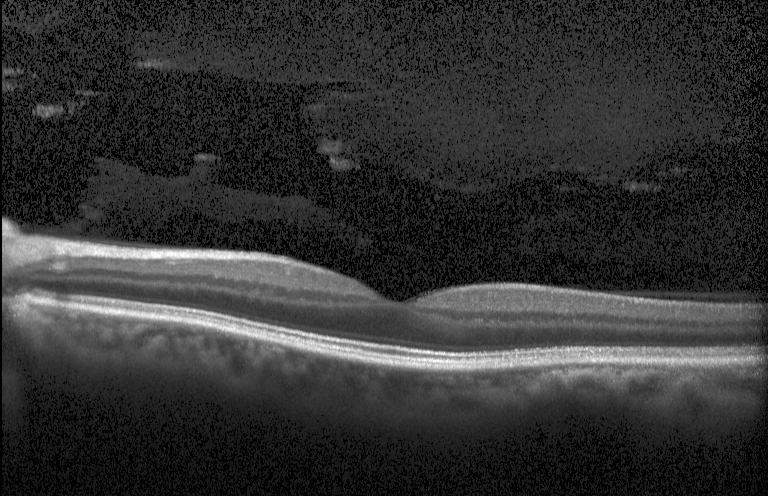
Assessment: no CNV, no DME, and no drusen.